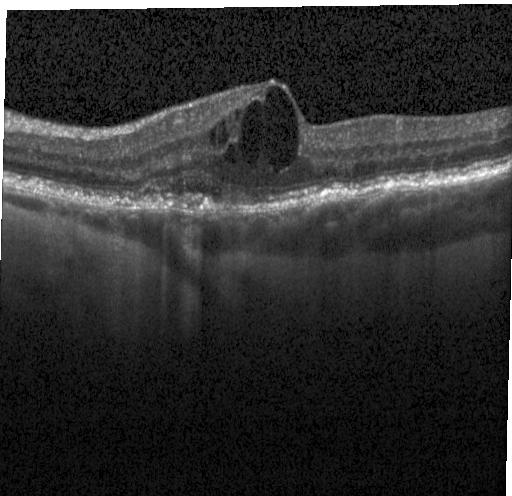
Retinal OCT B-scan; horizontal scan through the fovea; Heidelberg Spectralis OCT system; SD-OCT — A choroidal neovascular membrane.